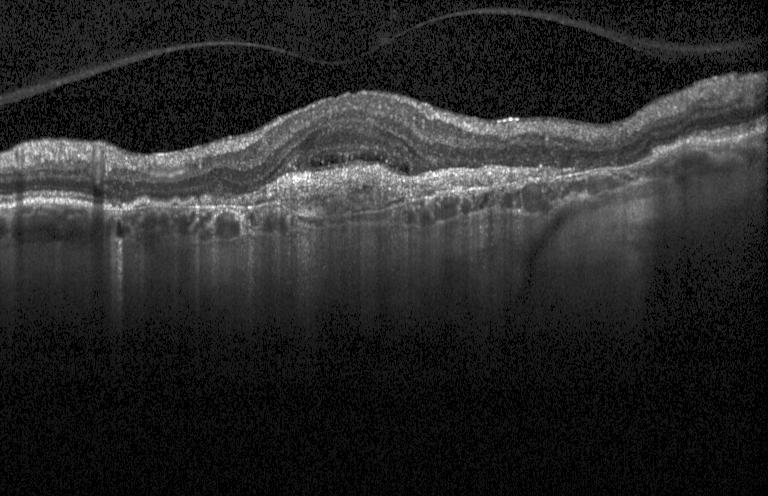 Horizontal scan through the fovea. Optical coherence tomography scan — The scan shows a choroidal neovascular membrane.